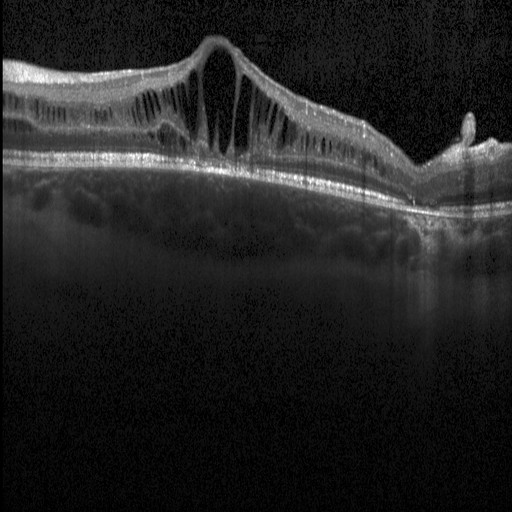 OCT B-scan.
The scan shows DME.